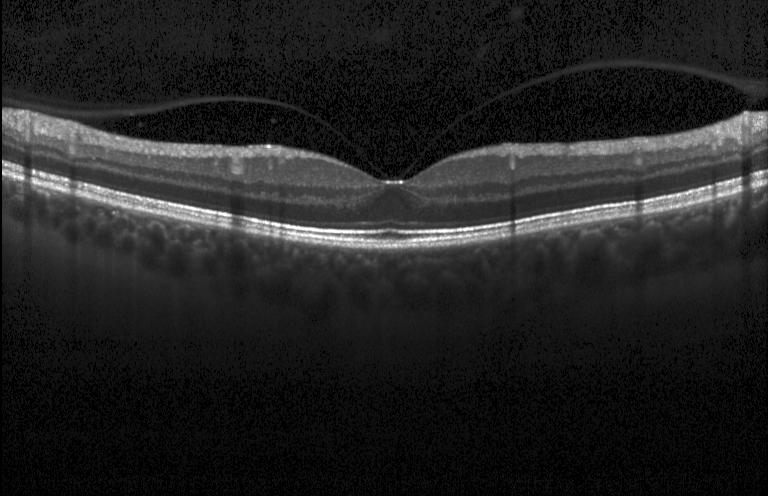 Spectral-domain OCT, through the macula, optical coherence tomography scan.
Macular OCT: neither choroidal neovascularization, diabetic macular edema, nor drusen.